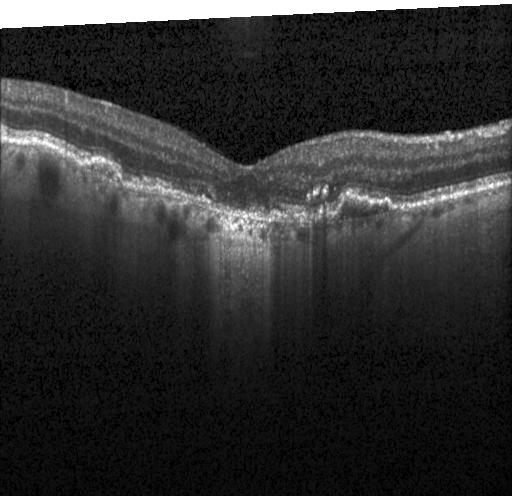

Macular OCT demonstrating choroidal neovascularization.